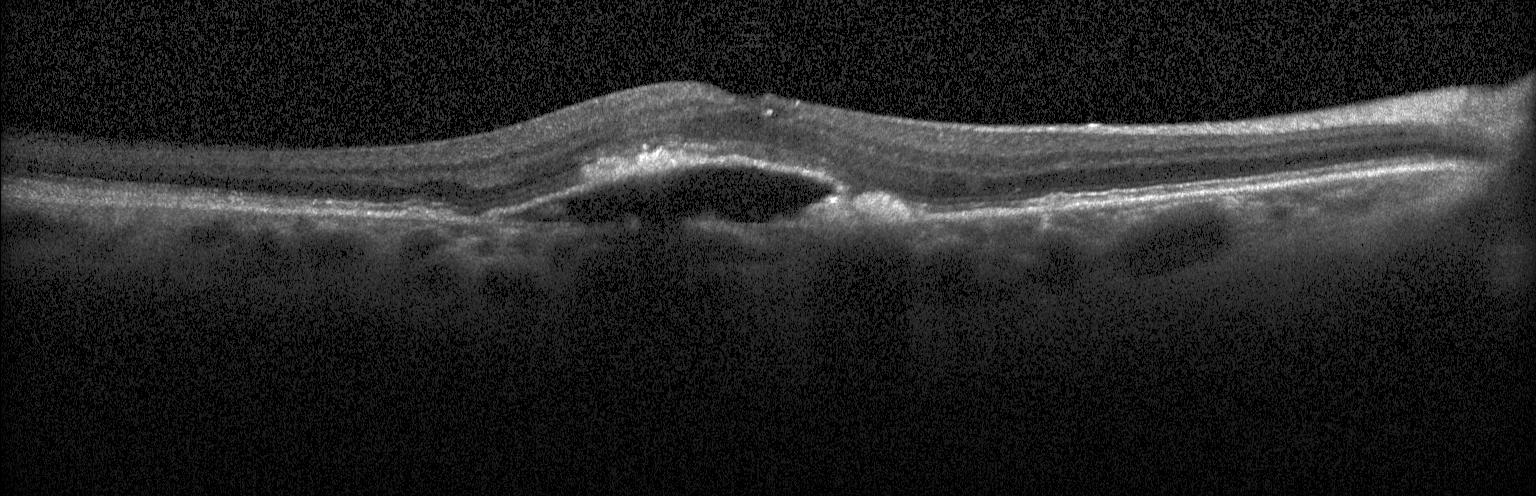 Optical coherence tomography B-scan
Macular OCT: CNV.